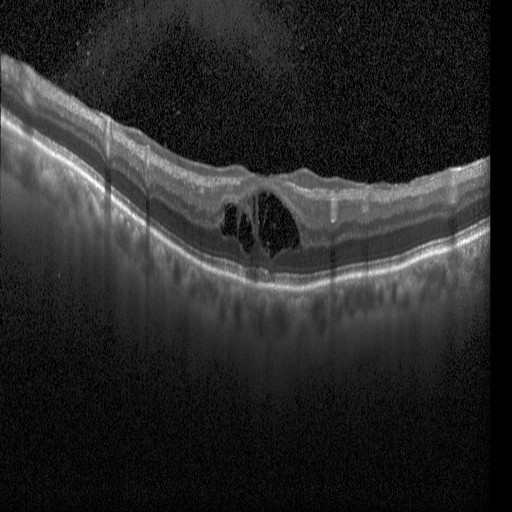 Spectral-domain optical coherence tomography, Heidelberg Spectralis, retinal OCT B-scan. Diagnosis: DME.